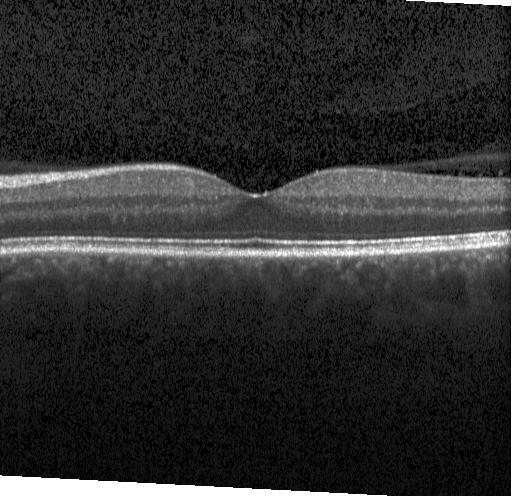

Through the macula · spectral-domain OCT · optical coherence tomography B-scan · Heidelberg Spectralis OCT system — Diagnosis: neither choroidal neovascularization, diabetic macular edema, nor drusen.